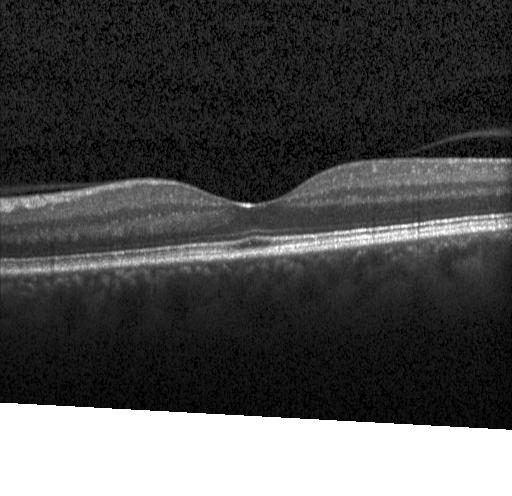
Retinal OCT cross-section, macular scan, SD-OCT, Heidelberg Spectralis OCT system — This B-scan demonstrates no evidence of choroidal neovascularization, diabetic macular edema, or drusen.